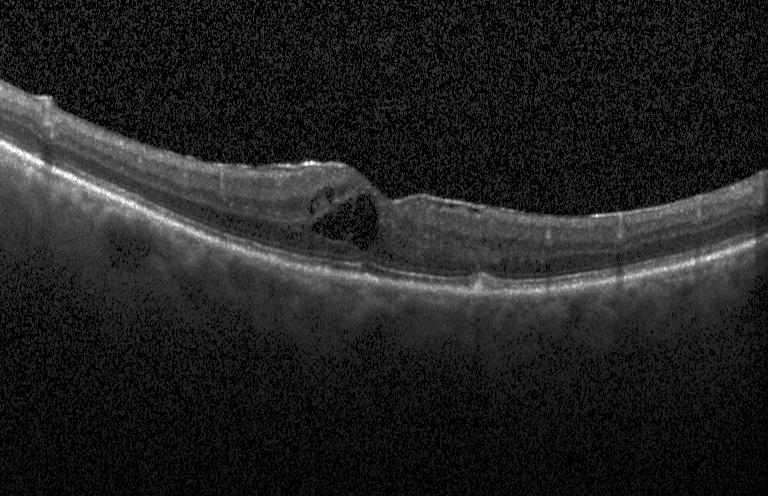

OCT B-scan, spectral-domain optical coherence tomography, centered on the fovea, Heidelberg Spectralis OCT system.
Diagnosis: diabetic macular edema.